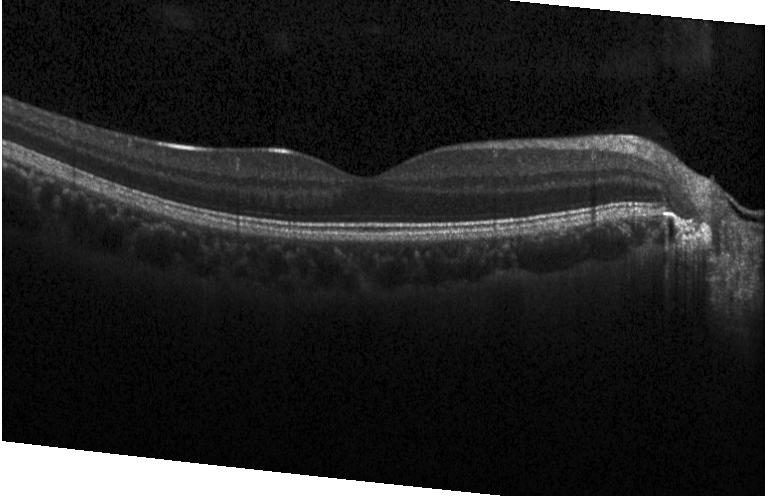
Heidelberg Spectralis OCT system, retinal OCT B-scan. The scan shows no choroidal neovascularization, diabetic macular edema, or drusen.